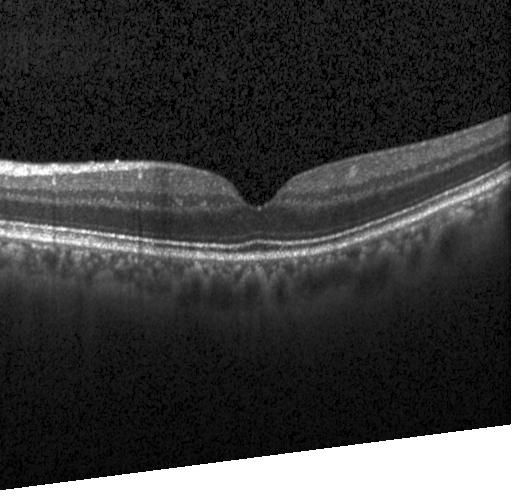

Retinal OCT cross-section showing no choroidal neovascularization, no diabetic macular edema, and no drusen.